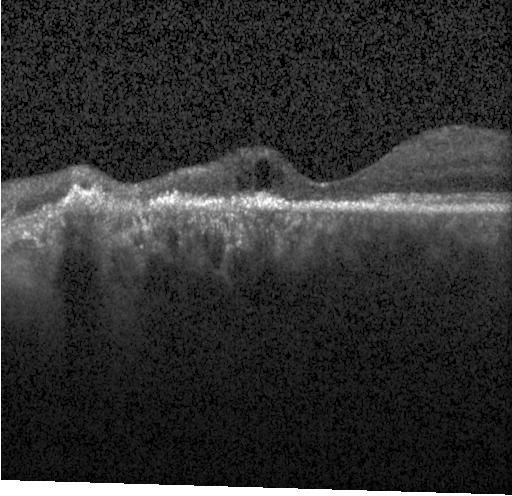

Diagnosis: a choroidal neovascular membrane.